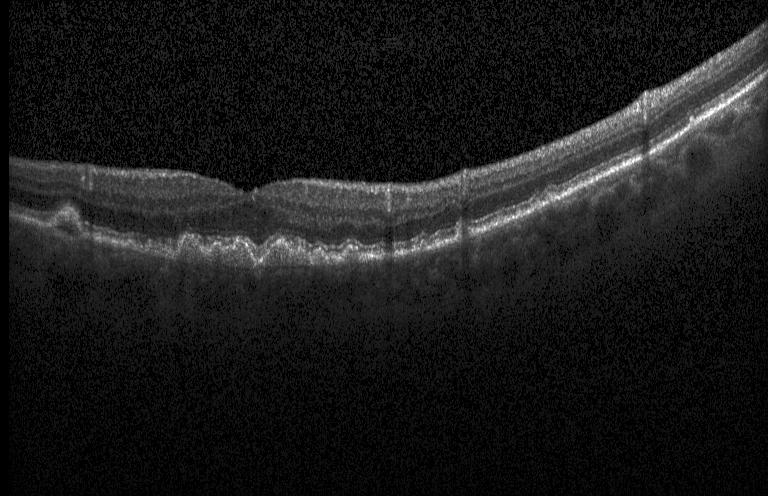

Optical coherence tomography B-scan
Impression: drusen.